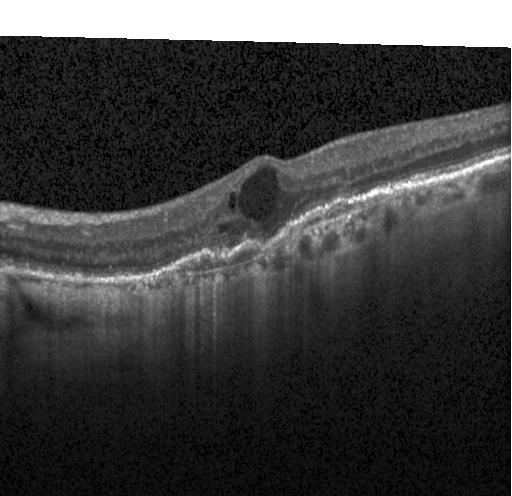 Assessment: choroidal neovascularization.